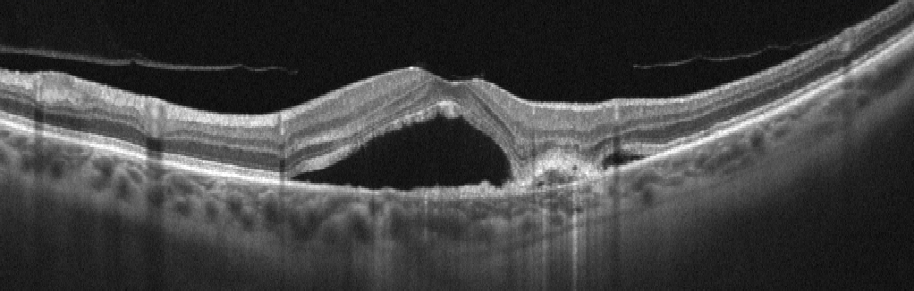 Optical coherence tomography B-scan · oculus sinister · macular scan · instrument: Optovue Avanti RTVue XR — OCT finding: age-related macular degeneration.